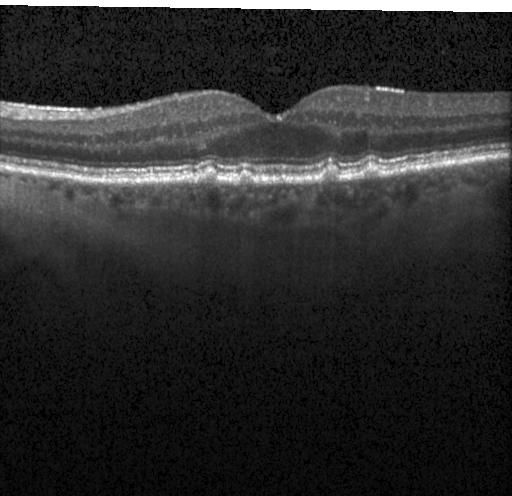
The scan shows sub-RPE drusenoid deposits.